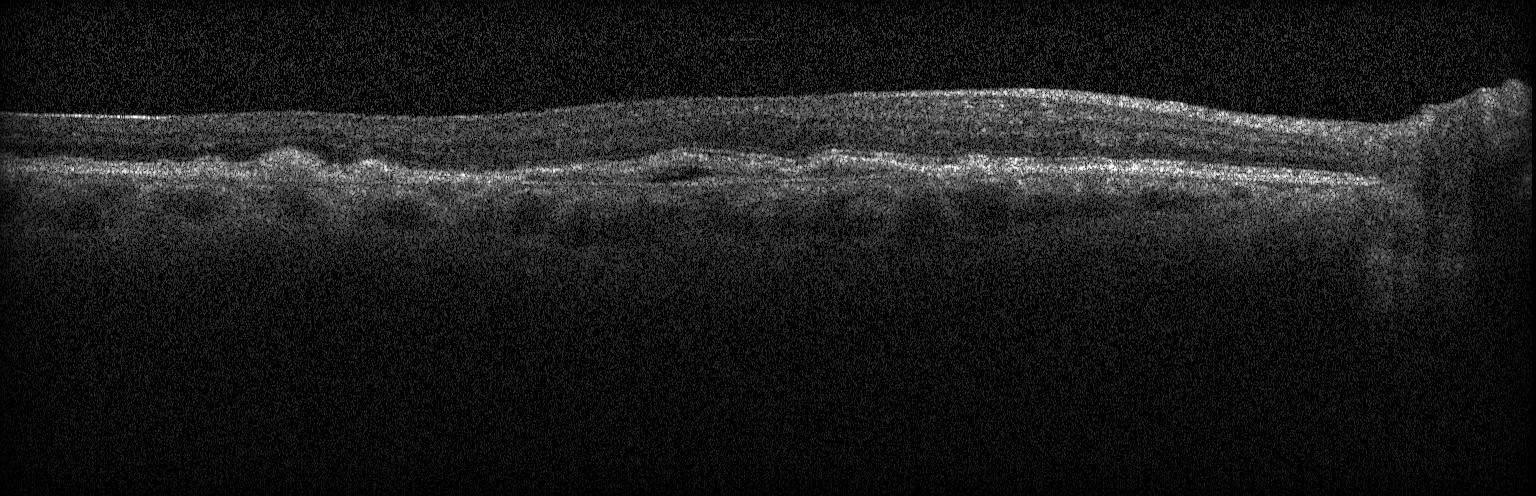
Spectral-domain OCT. OCT line scan. Fovea-centered.
This B-scan demonstrates a choroidal neovascular membrane.